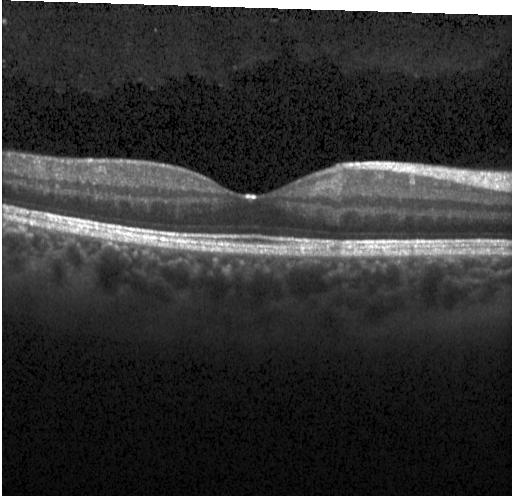

Impression: no evidence of choroidal neovascularization, diabetic macular edema, or drusen.